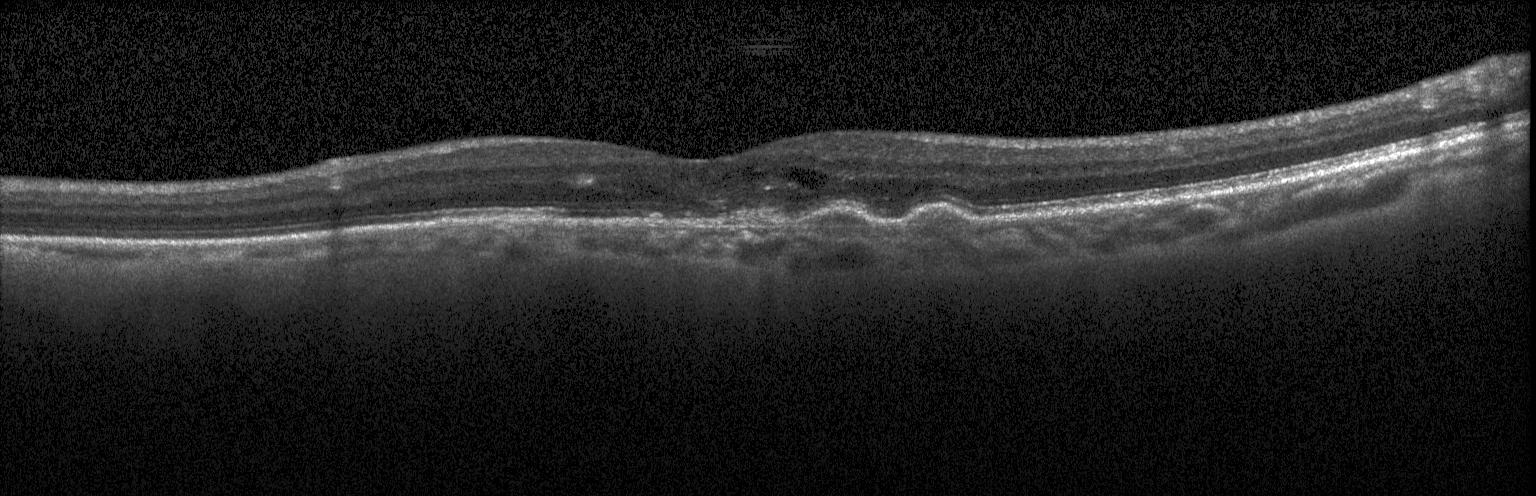
Retinal OCT B-scan · horizontal scan through the fovea · spectral-domain optical coherence tomography — Dx: CNV.